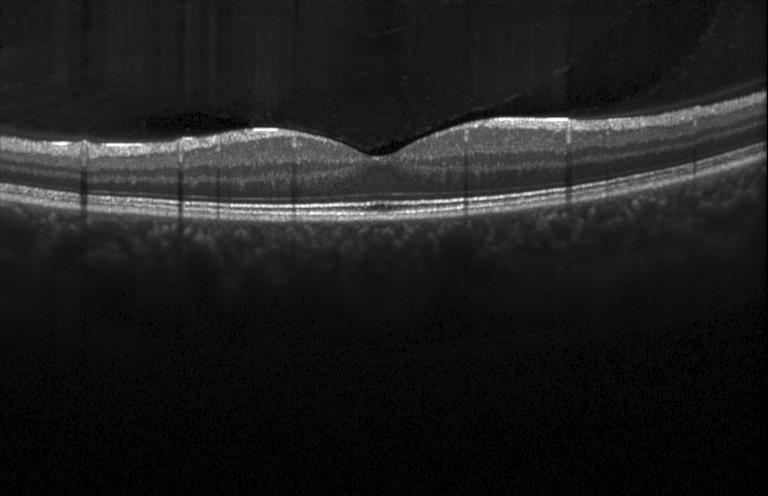
Neither CNV, DME, nor drusen.